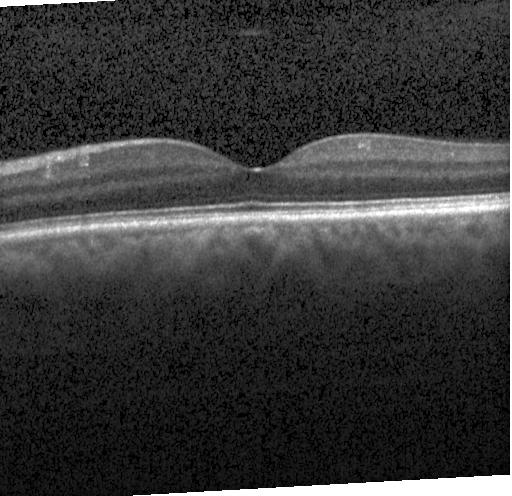
Dx: no choroidal neovascularization, no diabetic macular edema, and no drusen.